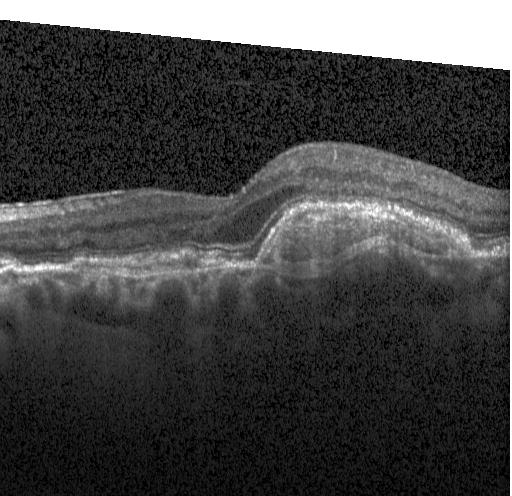

OCT finding: choroidal neovascularization.